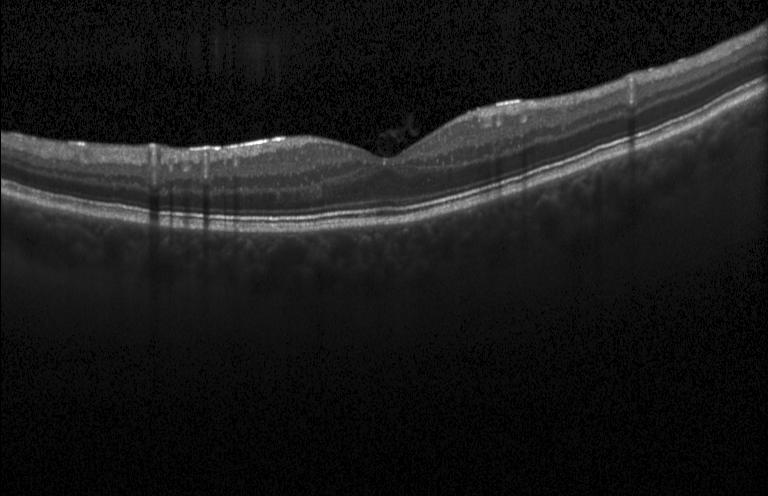

Optical coherence tomography B-scan. This B-scan demonstrates neither choroidal neovascularization, diabetic macular edema, nor drusen.